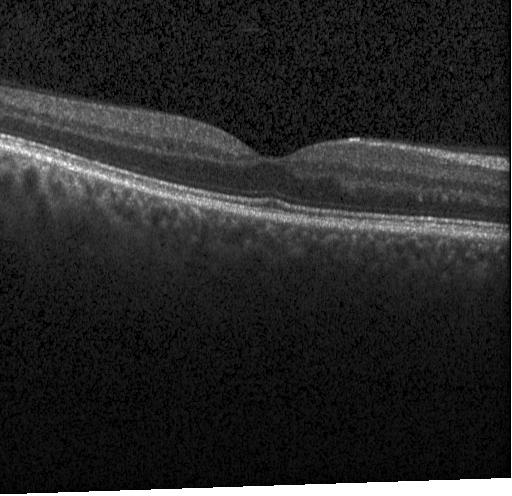

Fovea-centered; optical coherence tomography scan. Impression: no evidence of choroidal neovascularization, diabetic macular edema, or drusen.